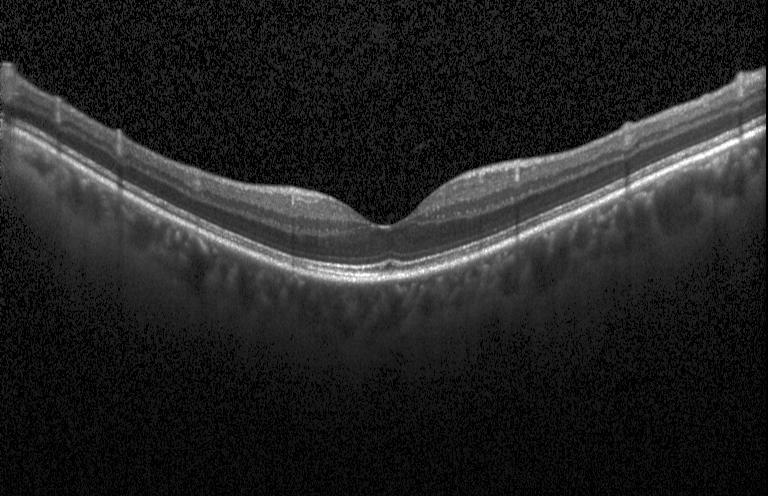
Diagnosis: no CNV, DME, or drusen.